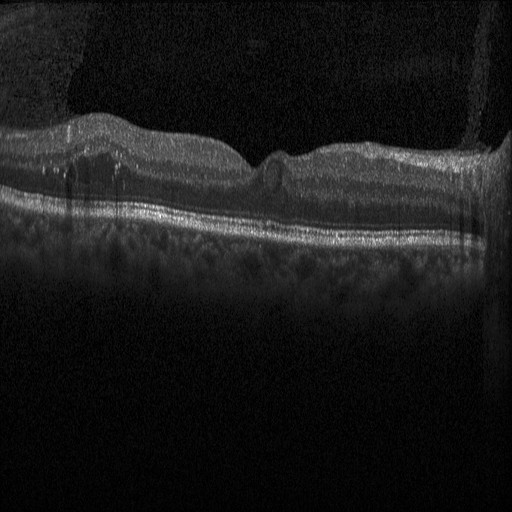 OCT finding: DME.